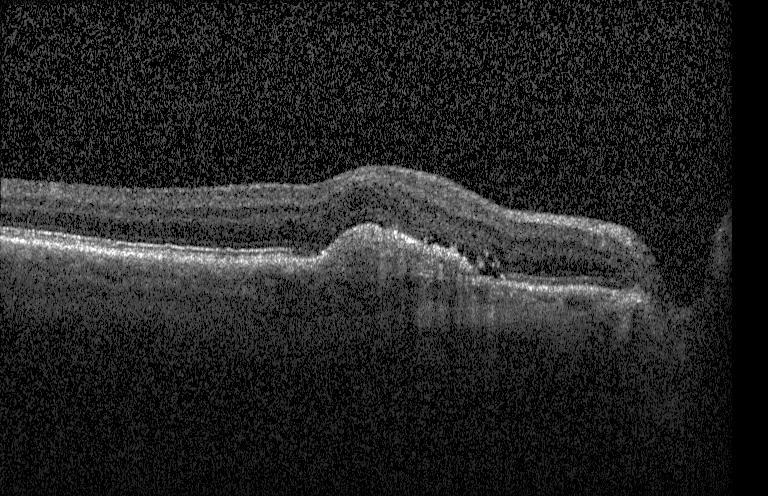

OCT scan showing choroidal neovascularization (CNV).